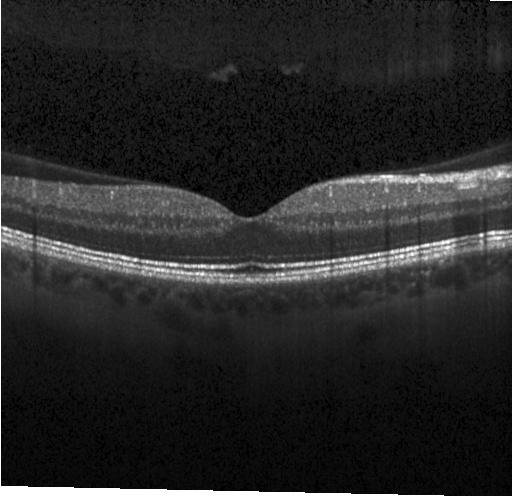

Centered on the fovea · OCT line scan. Impression: no choroidal neovascularization, diabetic macular edema, or drusen.